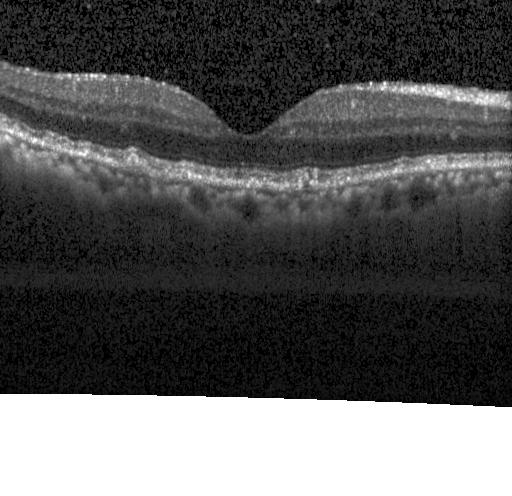 OCT line scan, Heidelberg Spectralis
Macular OCT: drusen.